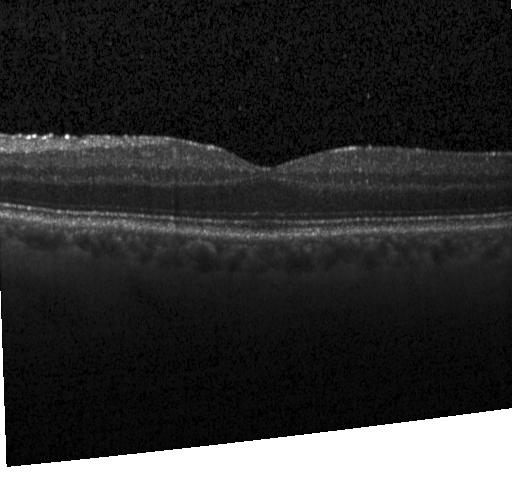 Spectral-domain OCT B-scan: no CNV, DME, or drusen.